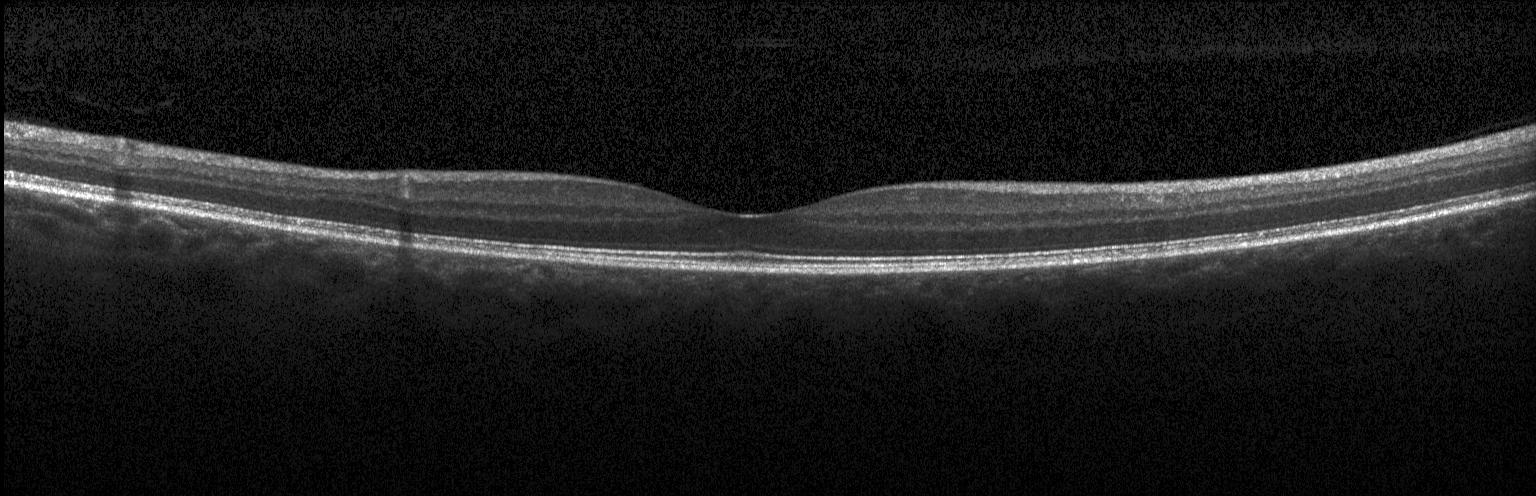

Dx: no evidence of CNV, DME, or drusen.